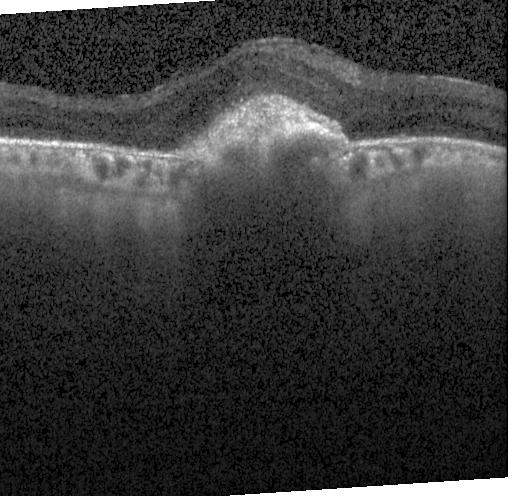

Optical coherence tomography B-scan; spectral-domain optical coherence tomography — Finding: a choroidal neovascular membrane.